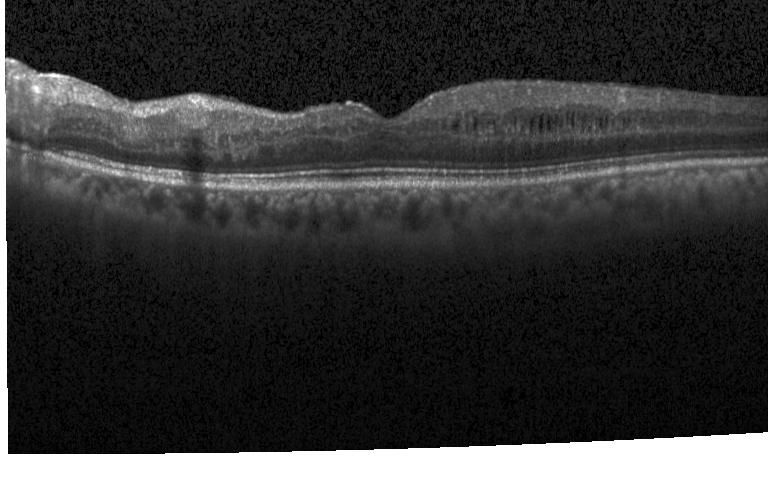
Fovea-centered; spectral-domain OCT; instrument: Heidelberg Spectralis; OCT B-scan.
Assessment: diabetic macular edema (DME).